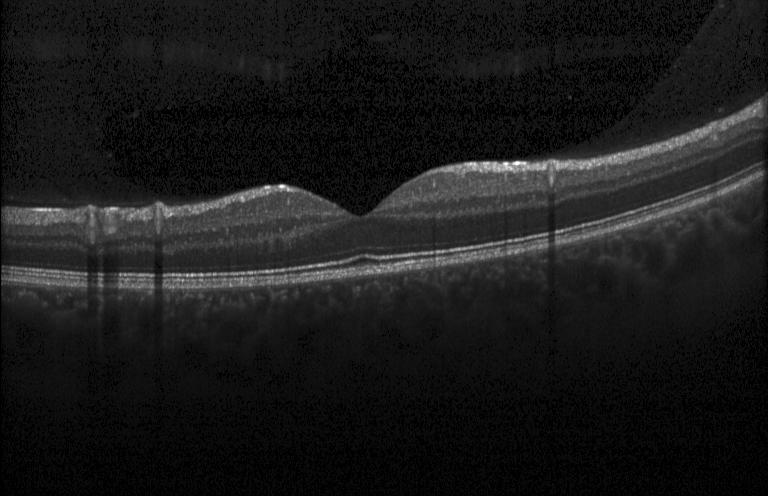
Diagnosis: neither choroidal neovascularization, diabetic macular edema, nor drusen.